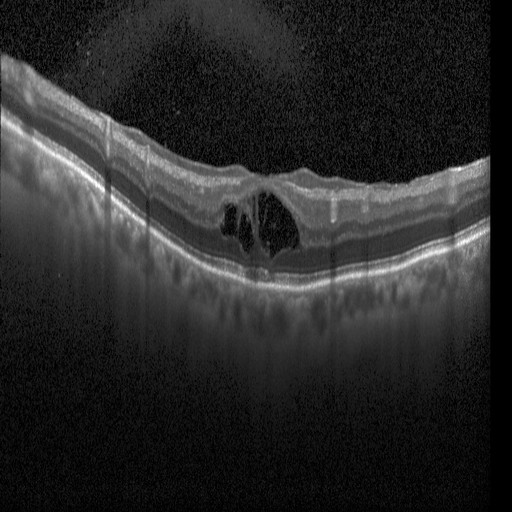
Finding: diabetic macular edema.